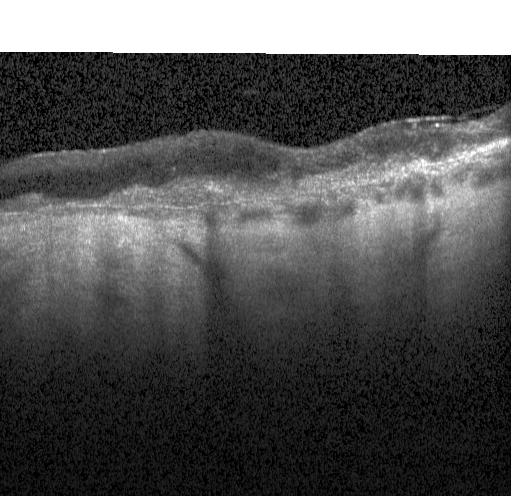
A choroidal neovascular membrane.